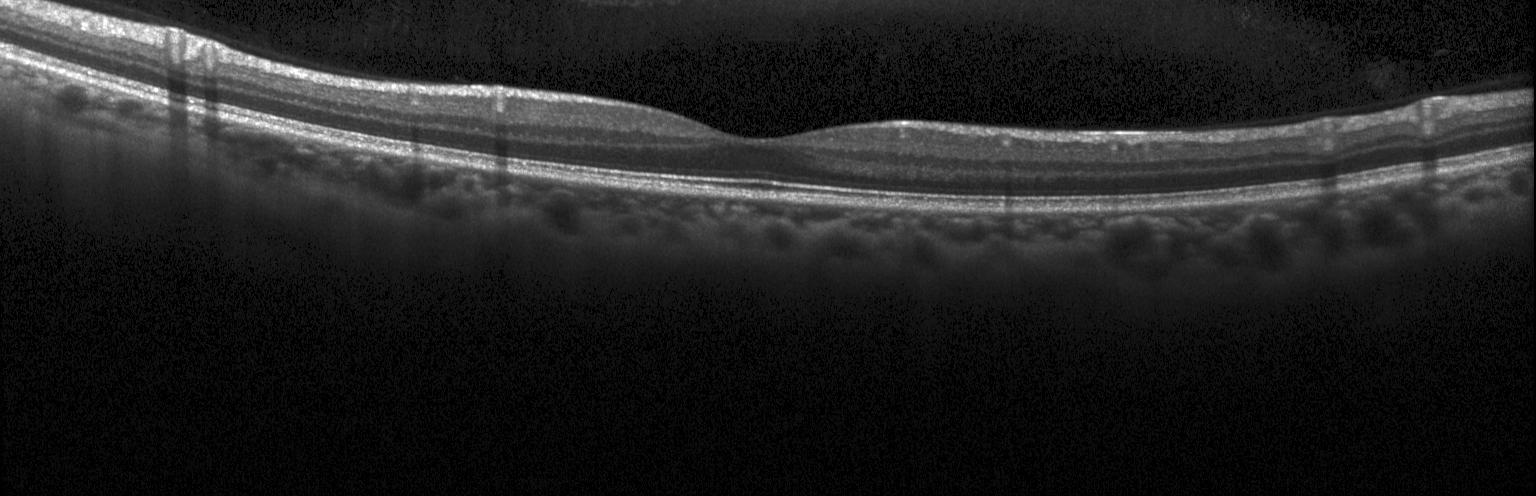
Fovea-centered, retinal OCT B-scan
Diagnosis: neither choroidal neovascularization, diabetic macular edema, nor drusen.